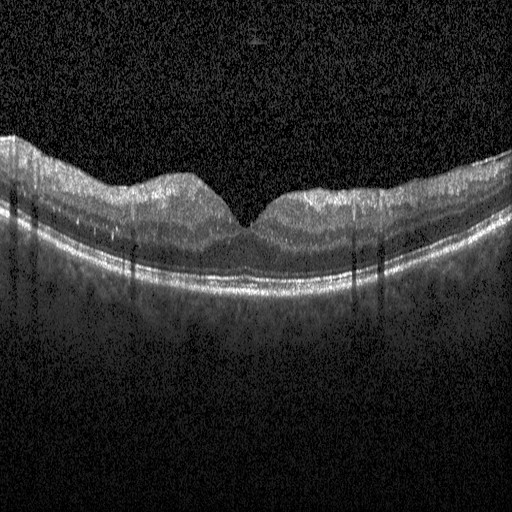

This B-scan demonstrates diabetic macular edema (DME).